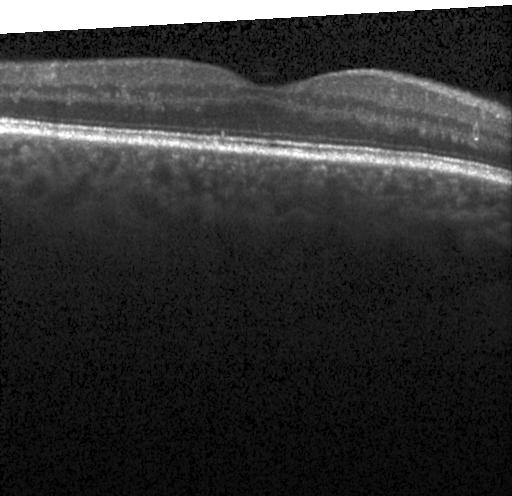

Heidelberg Spectralis; fovea-centered; spectral-domain OCT; OCT line scan. Diagnosis: no evidence of choroidal neovascularization, diabetic macular edema, or drusen.